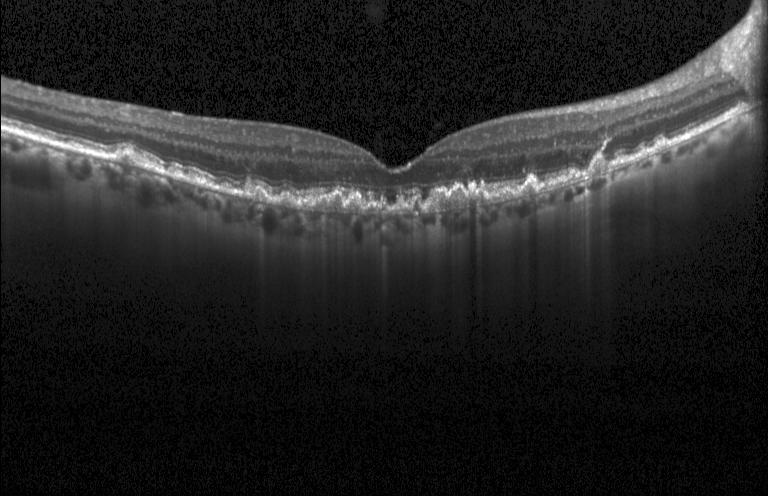

OCT line scan. OCT finding: sub-RPE drusenoid deposits.